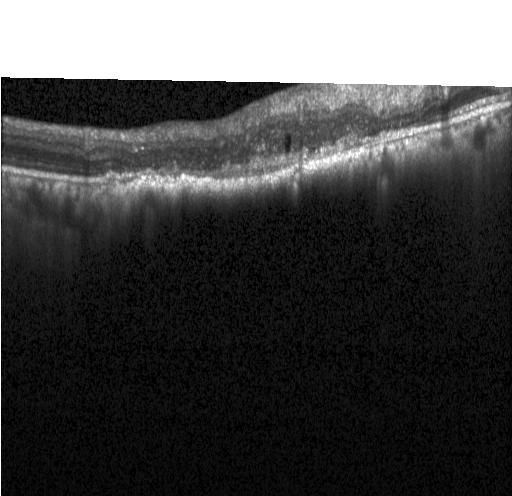 Optical coherence tomography scan. Impression: choroidal neovascularization.